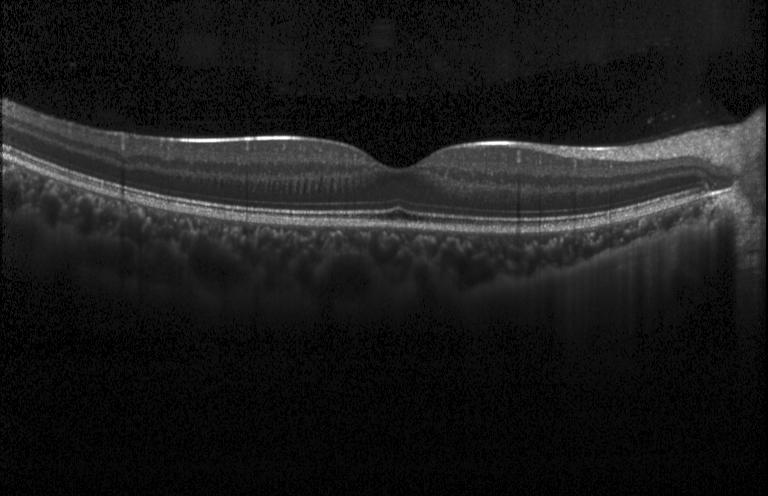
Assessment: no choroidal neovascularization, diabetic macular edema, or drusen.